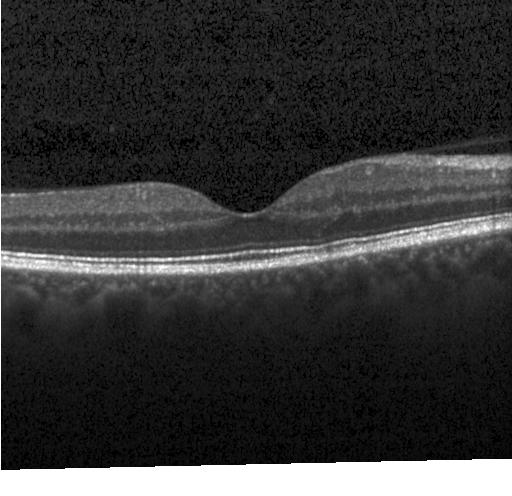
Retinal OCT cross-section showing no choroidal neovascularization, no diabetic macular edema, and no drusen.